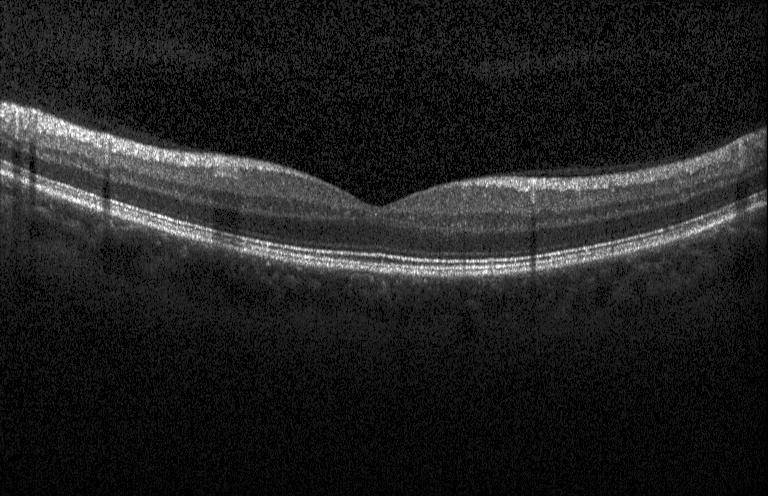

Heidelberg Spectralis · optical coherence tomography B-scan · centered on the fovea · SD-OCT — Diagnosis: no choroidal neovascularization, diabetic macular edema, or drusen.